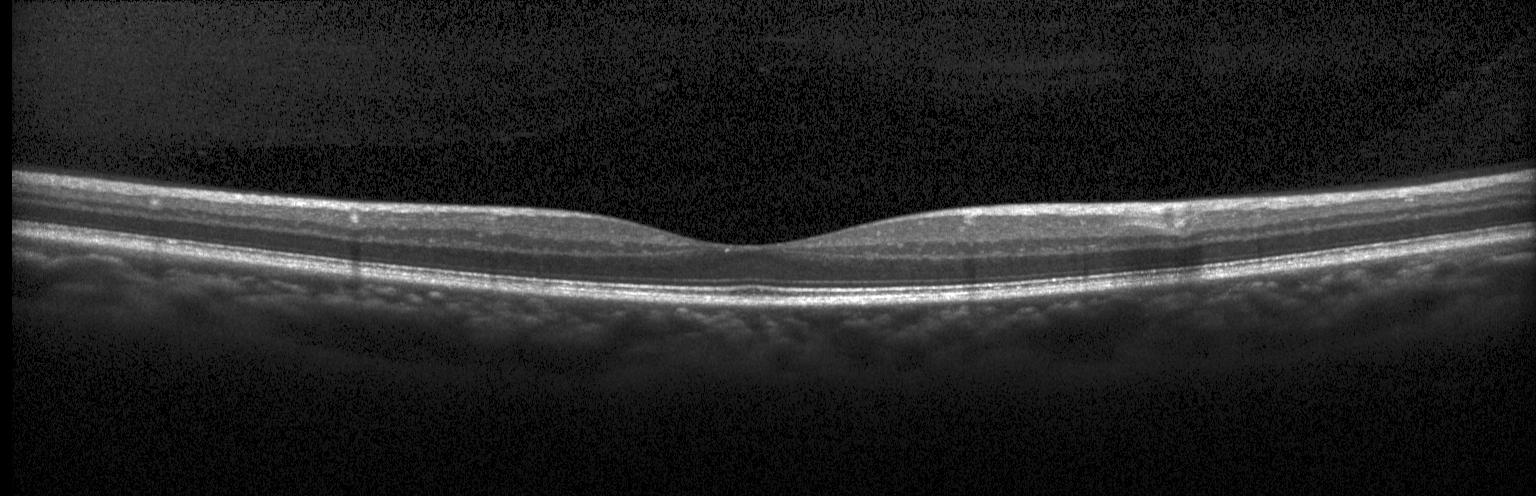
Diagnosis: neither choroidal neovascularization, diabetic macular edema, nor drusen.